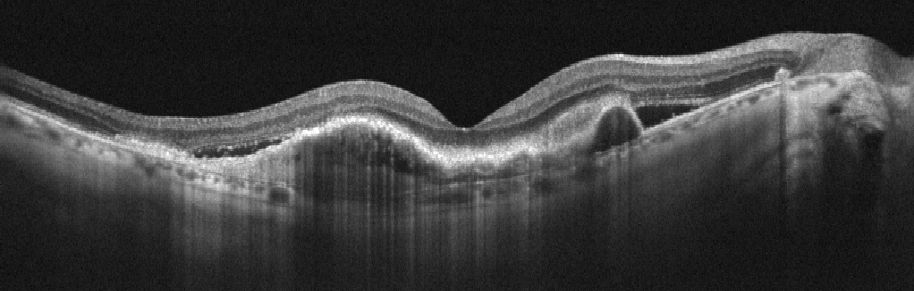
Oculus dexter, optical coherence tomography scan. This B-scan demonstrates age-related macular degeneration (AMD).